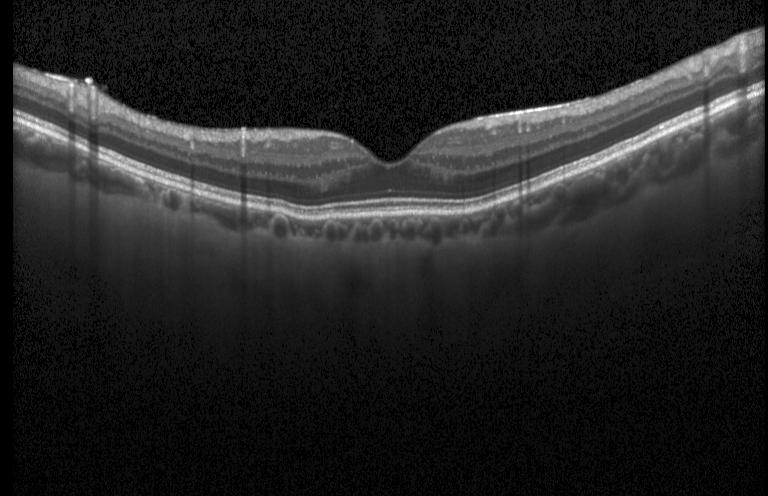
Diagnosis: no evidence of choroidal neovascularization, diabetic macular edema, or drusen.